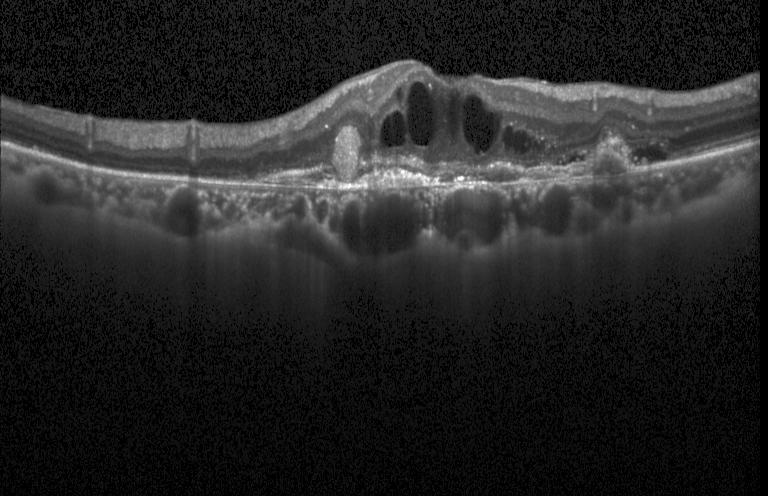 Retinal OCT cross-section.
A choroidal neovascular membrane.